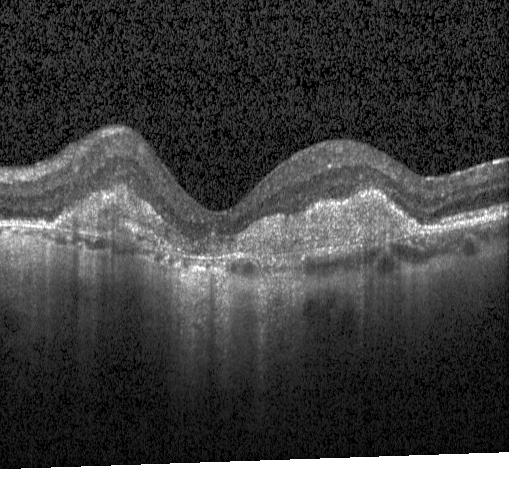 Macular scan; SD-OCT; Heidelberg Spectralis OCT system; optical coherence tomography B-scan — Diagnosis: a choroidal neovascular membrane.